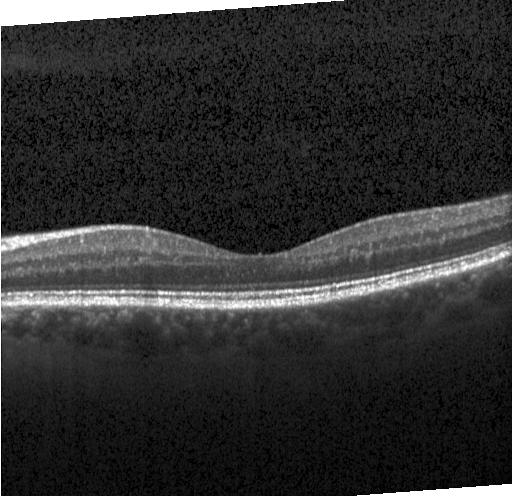 SD-OCT · through the macula · retinal OCT B-scan. Impression: no evidence of CNV, DME, or drusen.